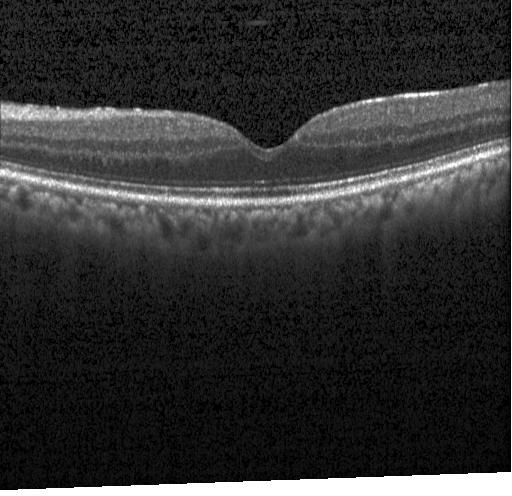
Through the macula; optical coherence tomography B-scan; instrument: Heidelberg Spectralis; spectral-domain optical coherence tomography
Dx: no evidence of choroidal neovascularization, diabetic macular edema, or drusen.